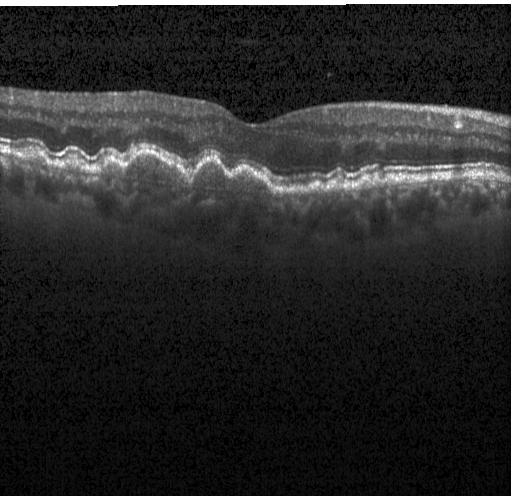
Through the macula · retinal OCT B-scan · SD-OCT
Diagnosis: drusen.